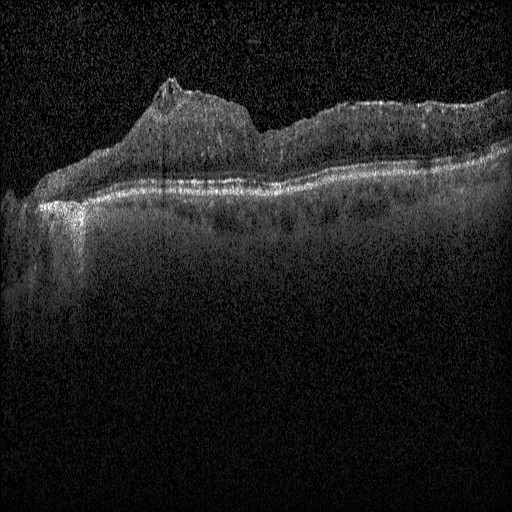
Retinal OCT B-scan.
Macular OCT: DME.